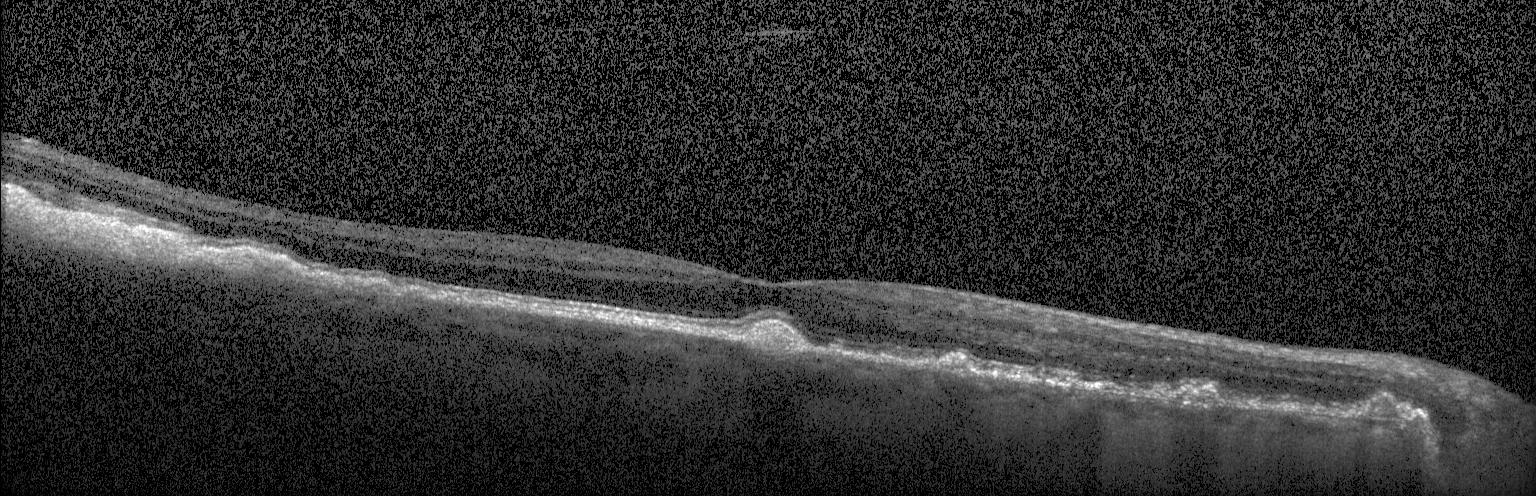
OCT finding: sub-RPE drusenoid deposits.